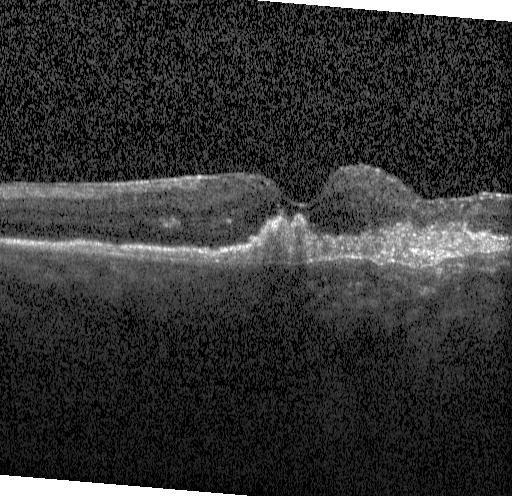 OCT finding: a choroidal neovascular membrane.